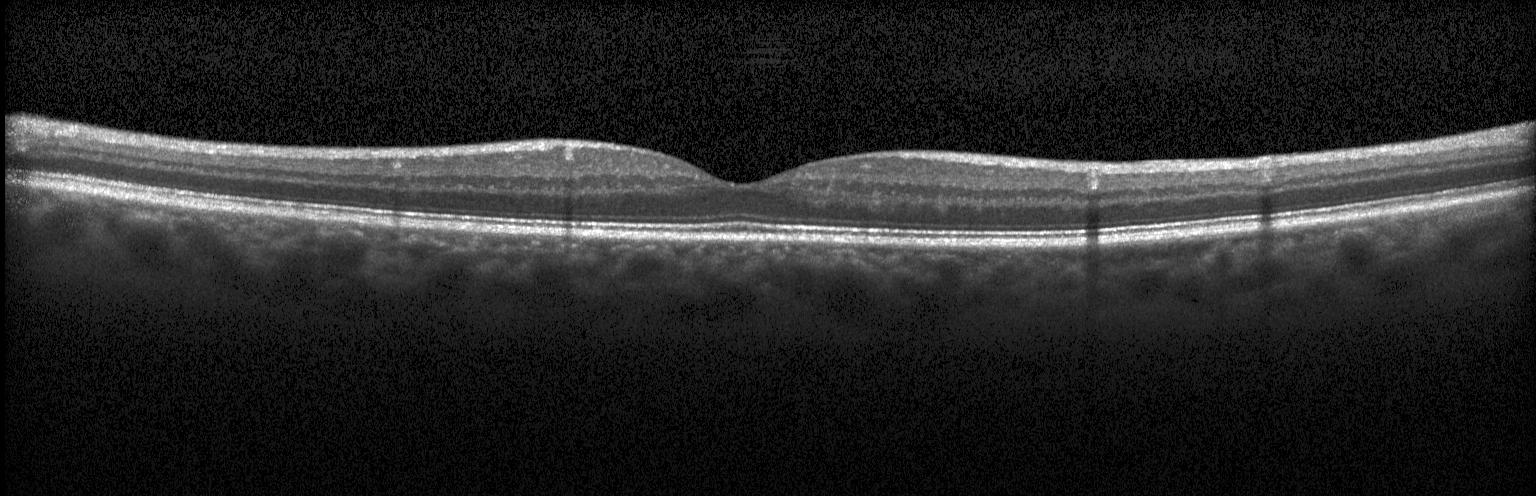

Optical coherence tomography B-scan
Assessment: no choroidal neovascularization, no diabetic macular edema, and no drusen.